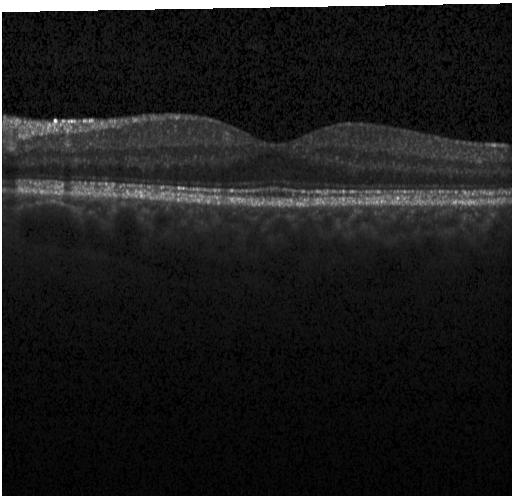
Macular scan · OCT line scan — OCT finding: no evidence of choroidal neovascularization, diabetic macular edema, or drusen.